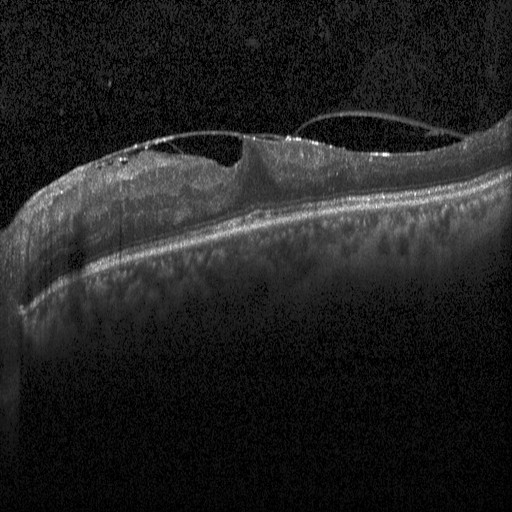
Diagnosis: DME.